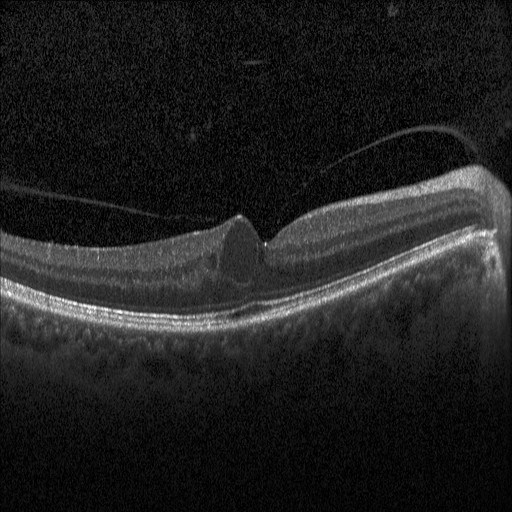
Retinal OCT cross-section — Impression: DME.